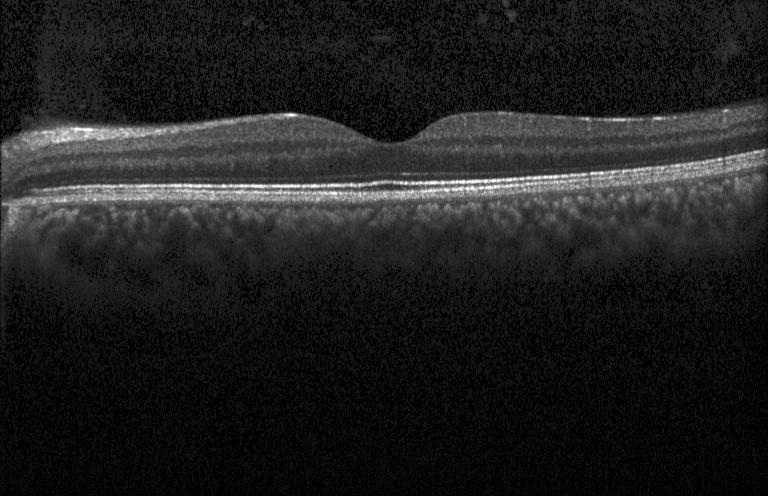

The scan shows neither choroidal neovascularization, diabetic macular edema, nor drusen.